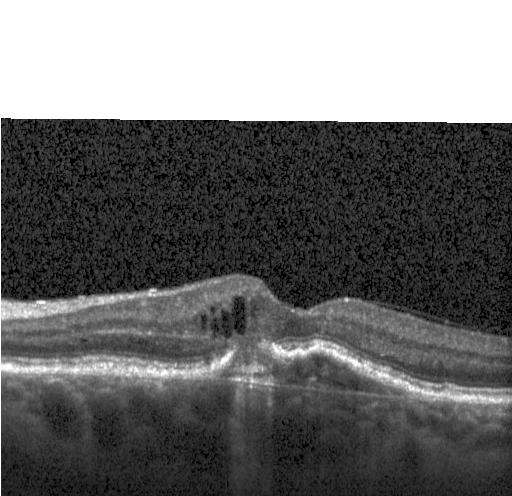
Spectral-domain optical coherence tomography; OCT line scan; fovea-centered.
Impression: a choroidal neovascular membrane.